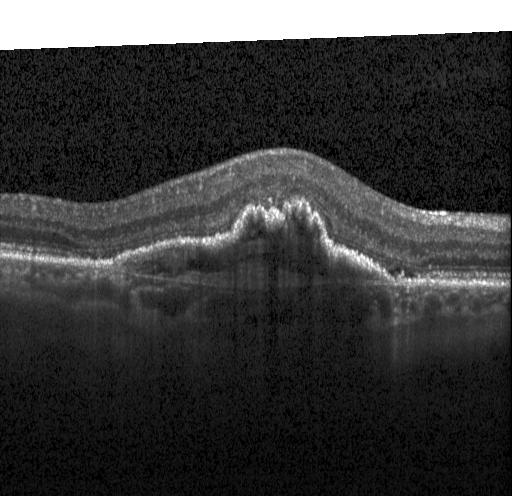

Macular OCT: choroidal neovascularization.